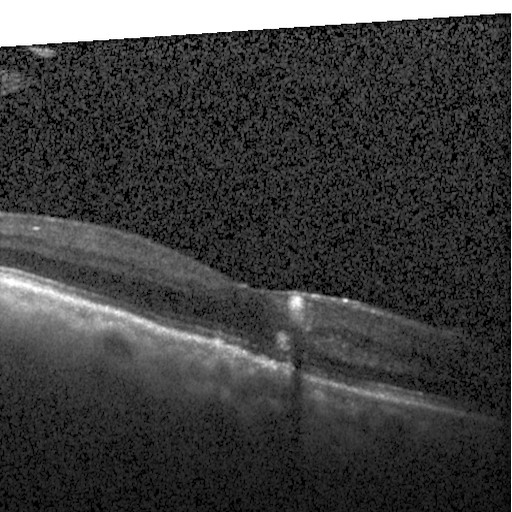 SD-OCT. Centered on the fovea. Retinal OCT cross-section — Finding: diabetic macular edema.